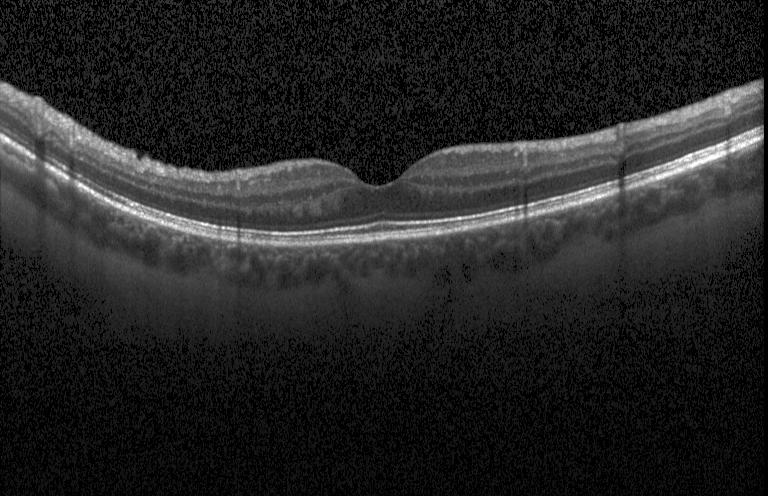
Diagnosis: neither CNV, DME, nor drusen.